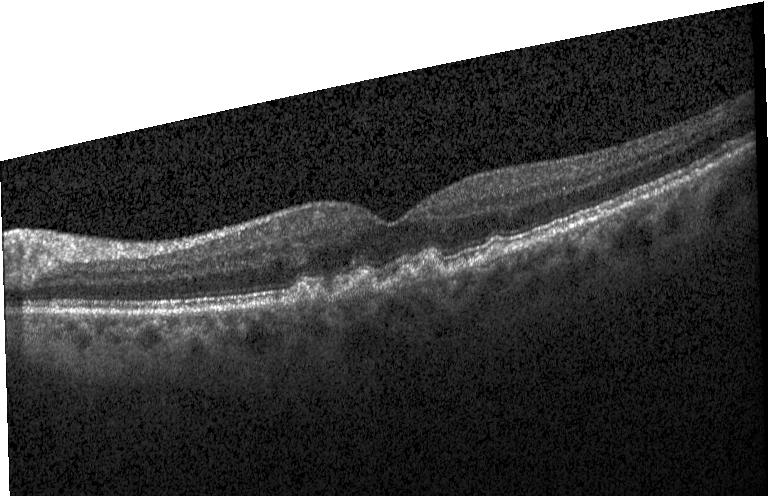 Retinal OCT cross-section; spectral-domain optical coherence tomography — Multiple drusen.